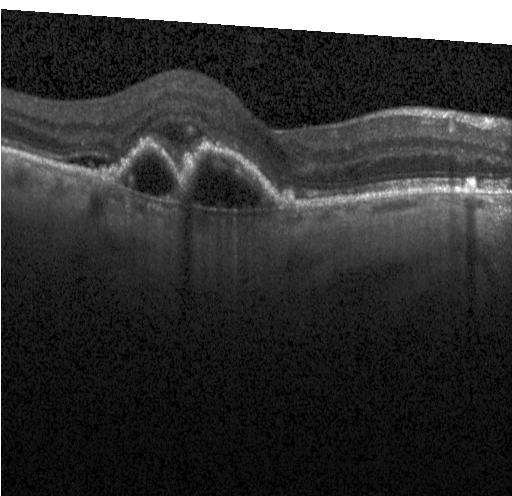
Macular OCT demonstrating a choroidal neovascular membrane.